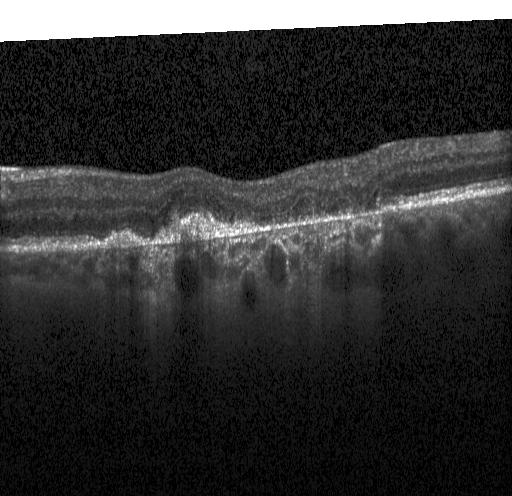 OCT finding: CNV.